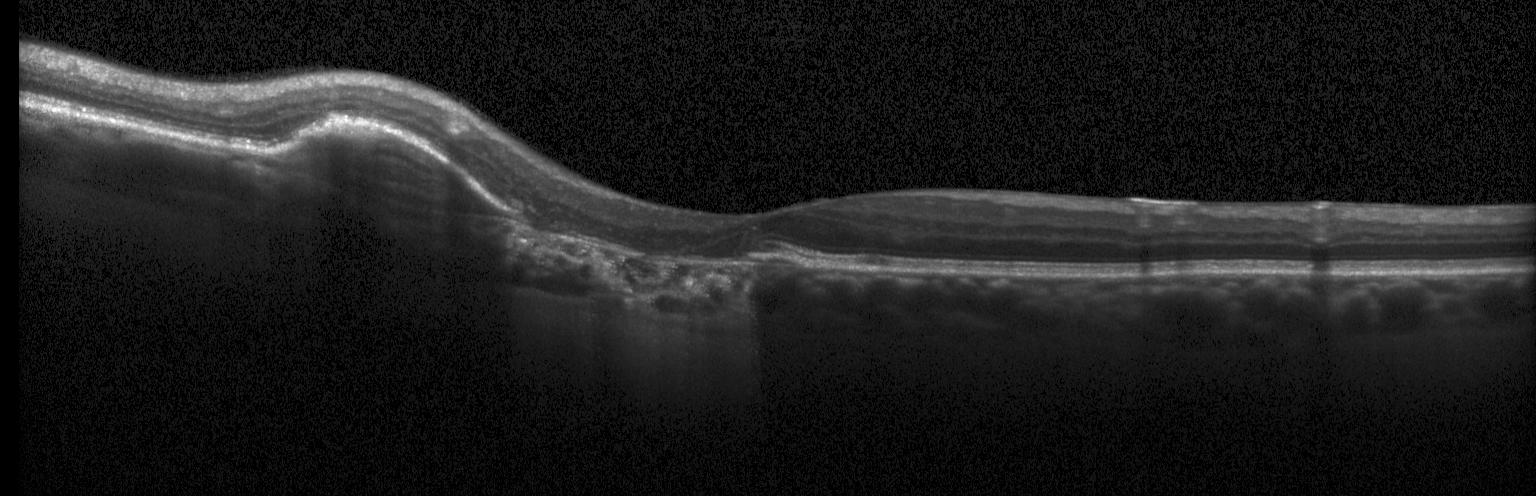 Diagnosis: CNV.